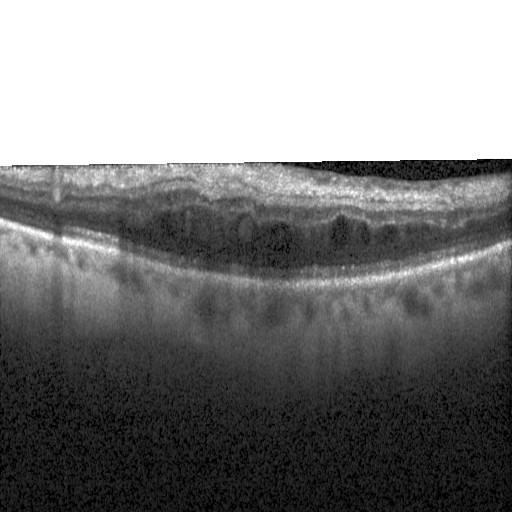 Centered on the fovea. Retinal OCT B-scan
Macular OCT: diabetic macular edema.